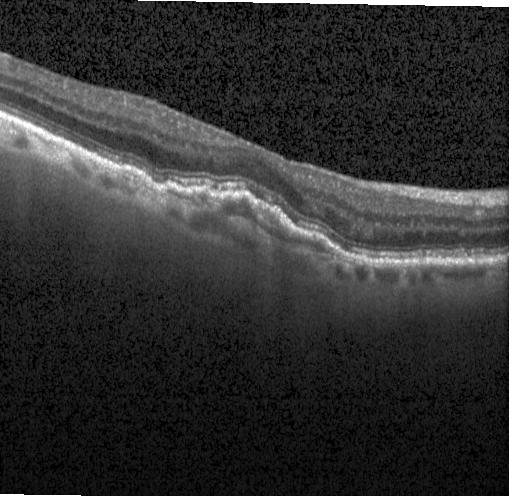

OCT B-scan. Spectral-domain OCT. Macular OCT: a choroidal neovascular membrane.